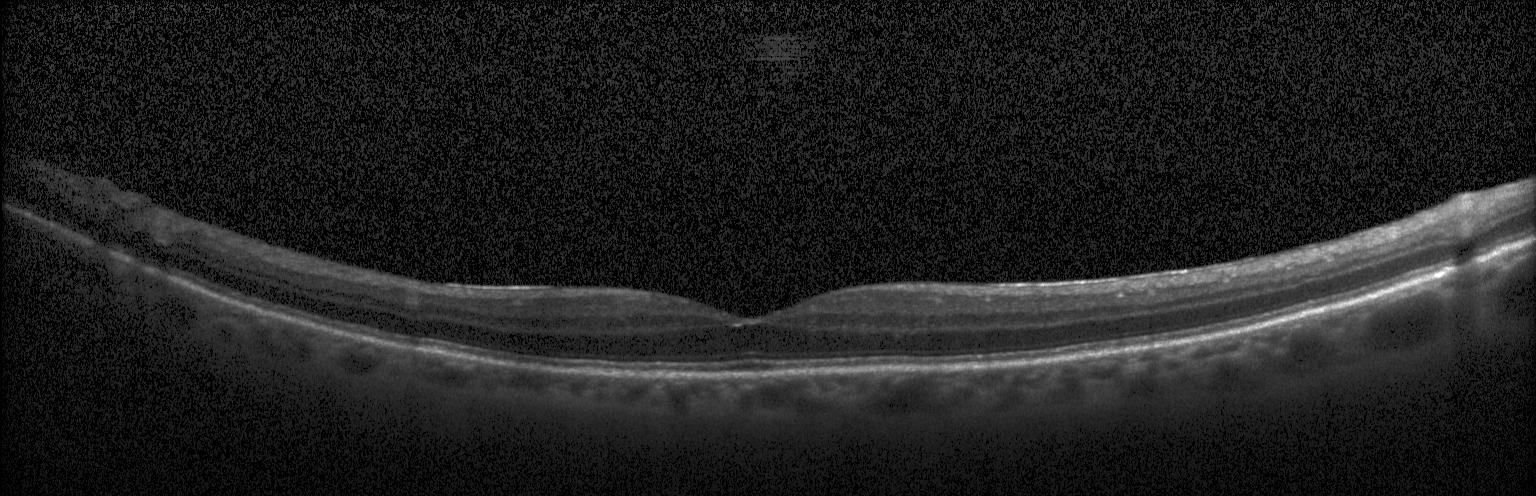
Macular OCT: neither CNV, DME, nor drusen.